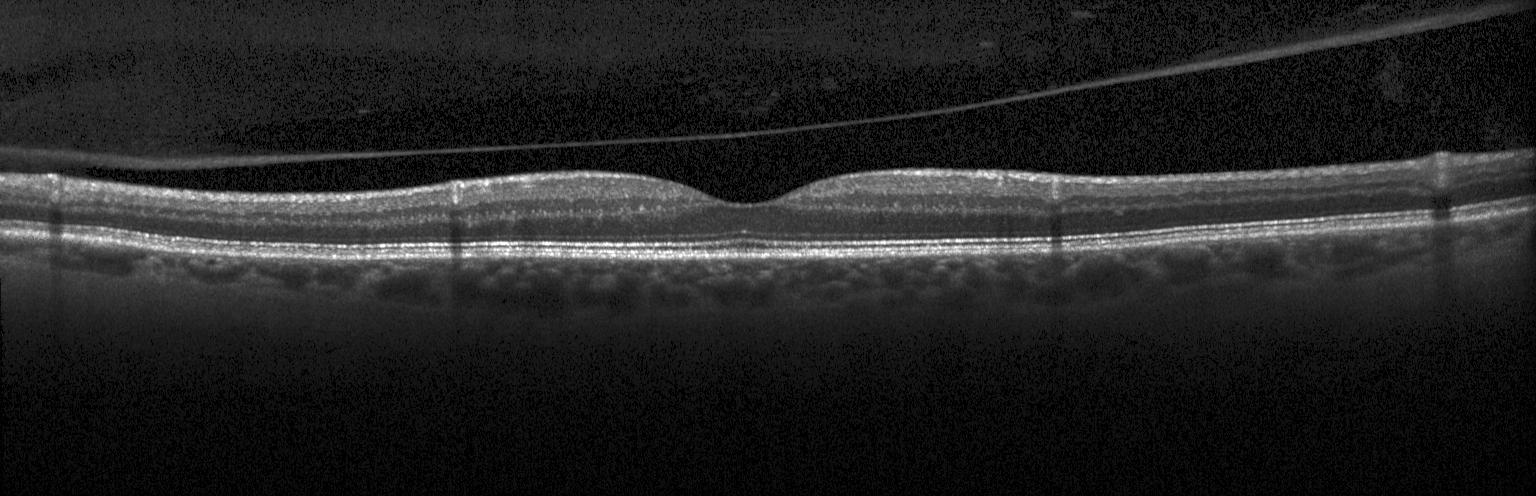
Dx: neither choroidal neovascularization, diabetic macular edema, nor drusen.